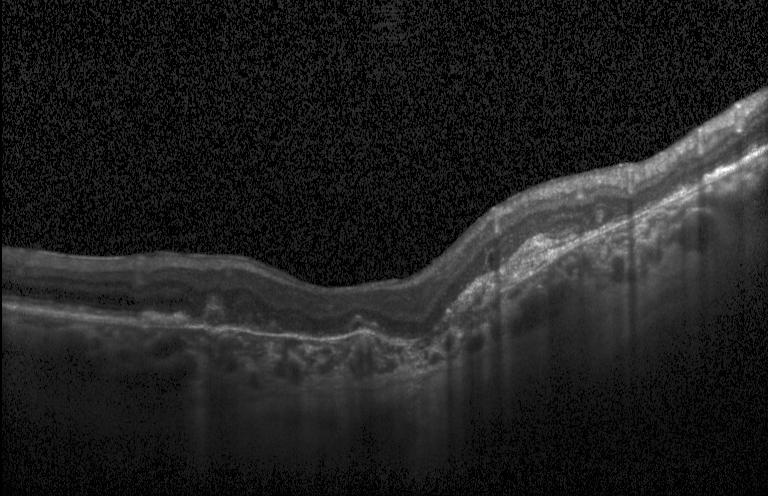

Acquired on a Heidelberg Spectralis. Through the macula. OCT line scan — Macular OCT: a choroidal neovascular membrane.